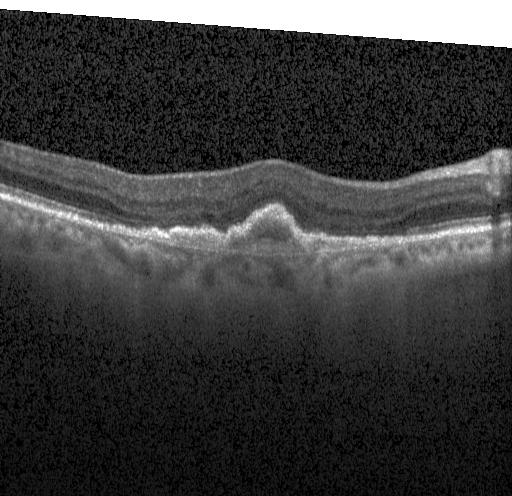

SD-OCT. Centered on the fovea. Optical coherence tomography B-scan
Macular OCT: CNV.